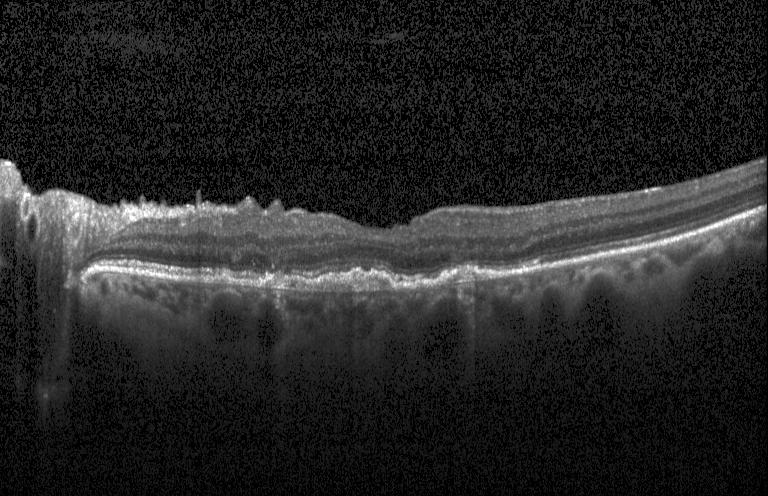
Retinal OCT cross-section
This B-scan demonstrates a choroidal neovascular membrane.